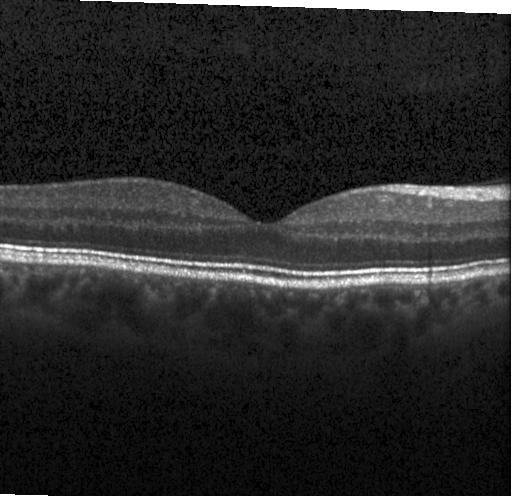 Retinal OCT B-scan · fovea-centered · SD-OCT · instrument: Heidelberg Spectralis — Impression: no evidence of choroidal neovascularization, diabetic macular edema, or drusen.